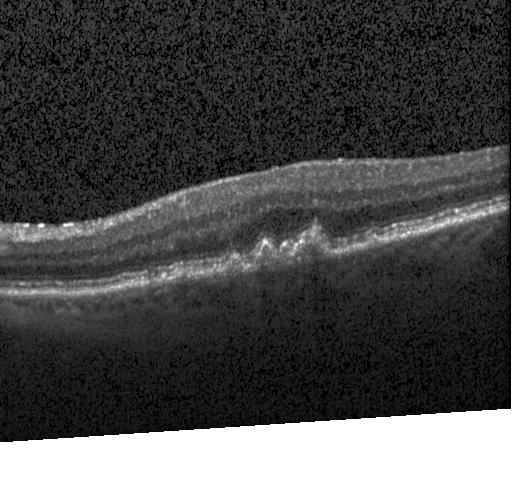 Retinal OCT cross-section showing sub-RPE drusenoid deposits.